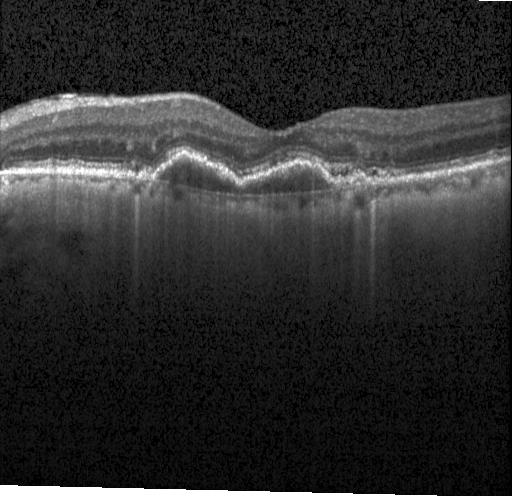 Spectral-domain optical coherence tomography · OCT B-scan.
Finding: a choroidal neovascular membrane.